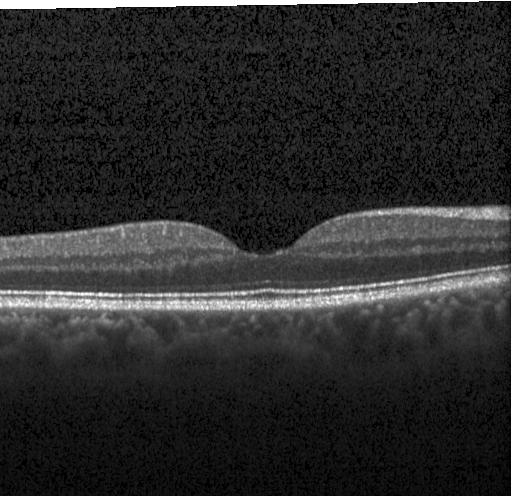
OCT line scan. Dx: no choroidal neovascularization, no diabetic macular edema, and no drusen.